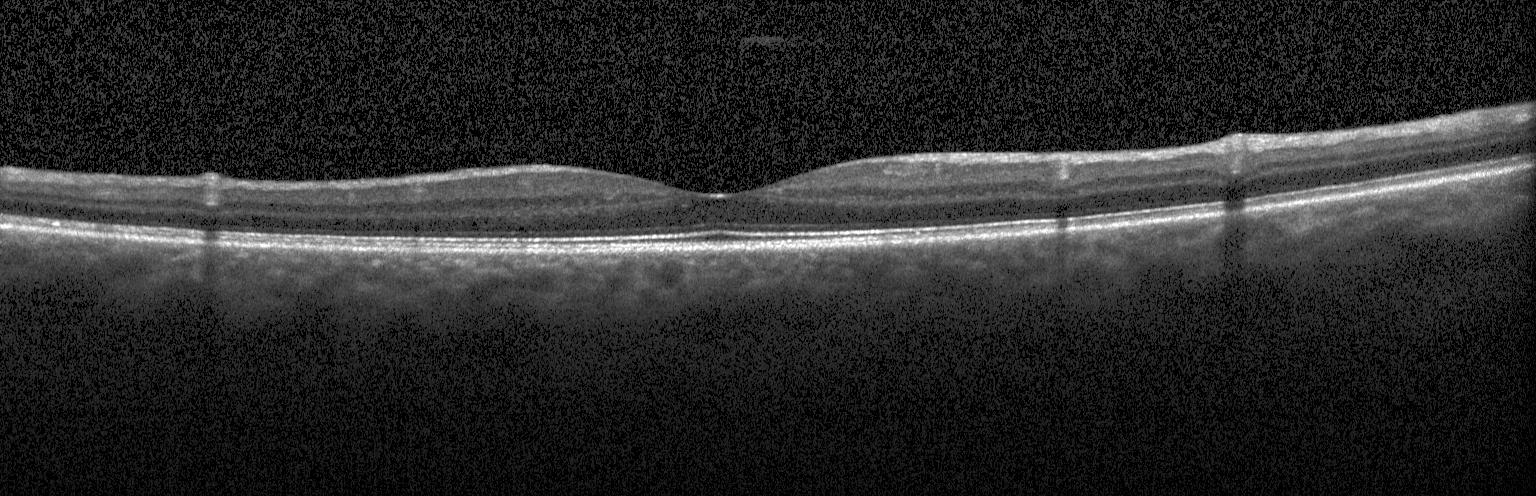
Retinal OCT cross-section. Heidelberg Spectralis. SD-OCT — OCT finding: no evidence of choroidal neovascularization, diabetic macular edema, or drusen.